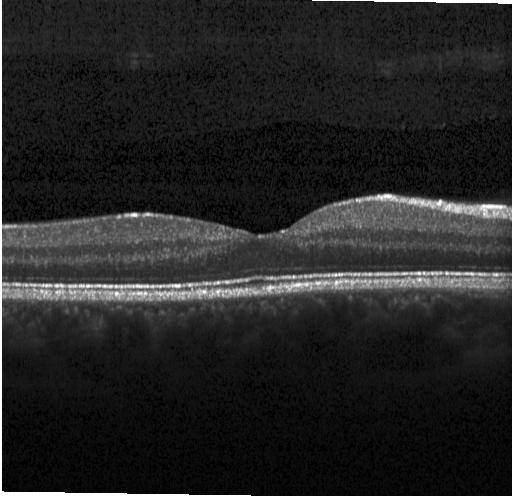
Retinal OCT cross-section; acquired on a Heidelberg Spectralis; SD-OCT; centered on the fovea — Dx: no evidence of CNV, DME, or drusen.